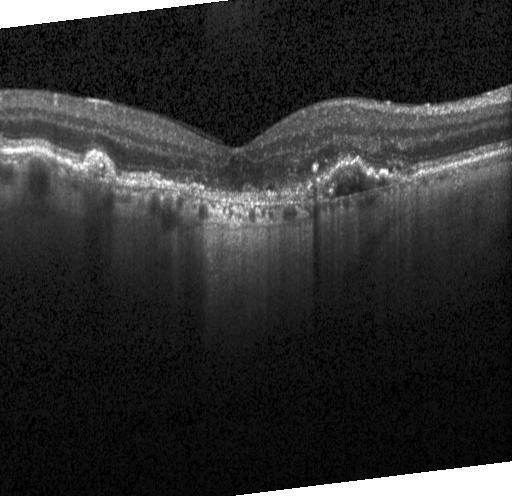
Macular OCT demonstrating choroidal neovascularization.